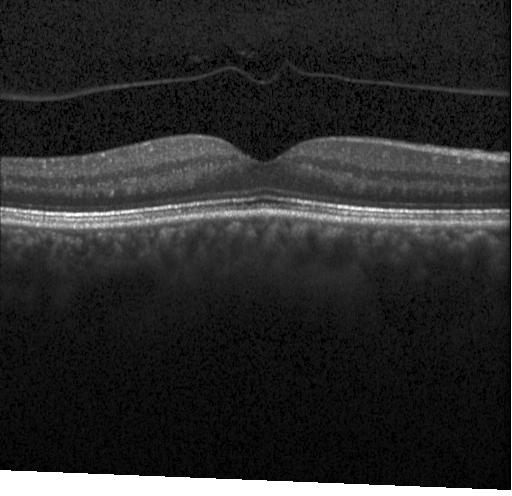

OCT B-scan · macular scan · Heidelberg Spectralis OCT system. Finding: no evidence of CNV, DME, or drusen.